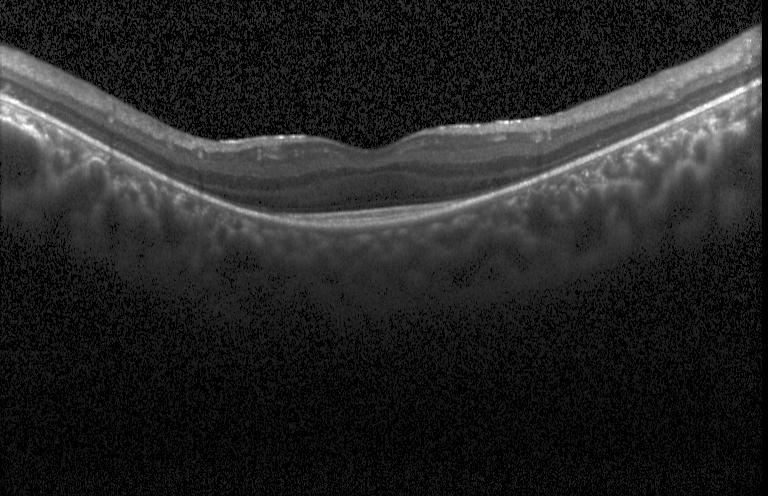 Heidelberg Spectralis OCT system. SD-OCT. OCT B-scan
OCT finding: neither choroidal neovascularization, diabetic macular edema, nor drusen.